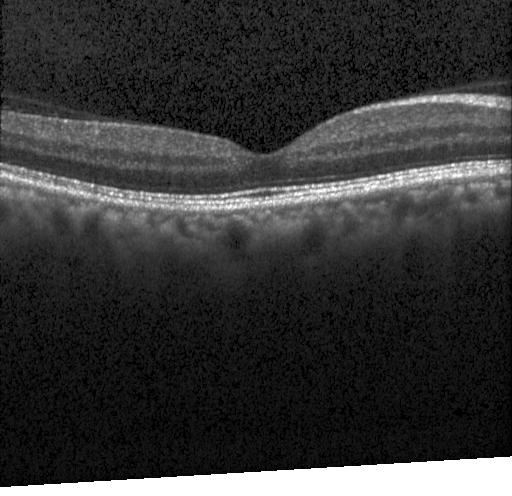

OCT finding: no evidence of choroidal neovascularization, diabetic macular edema, or drusen.